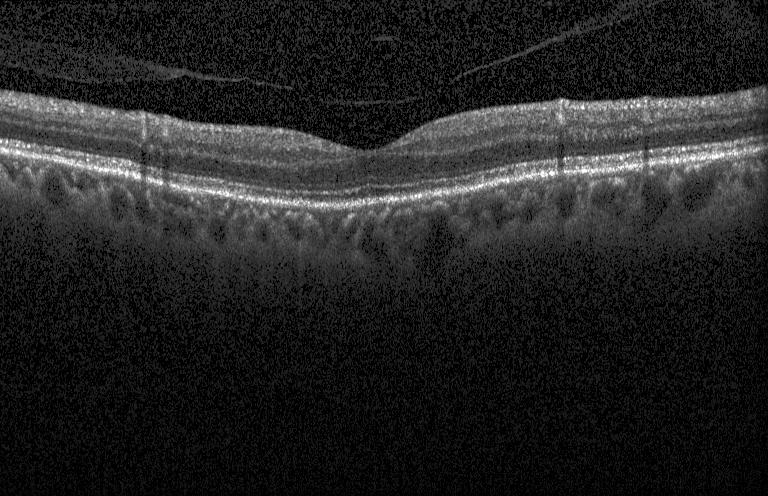
Macular scan. Optical coherence tomography B-scan — OCT finding: no CNV, DME, or drusen.